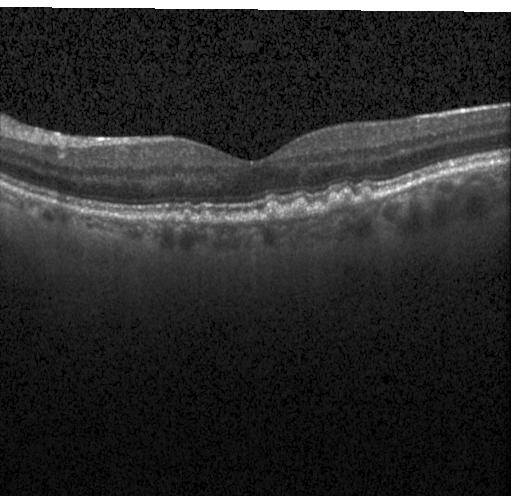 Spectral-domain OCT. Retinal OCT cross-section.
Finding: multiple drusen.